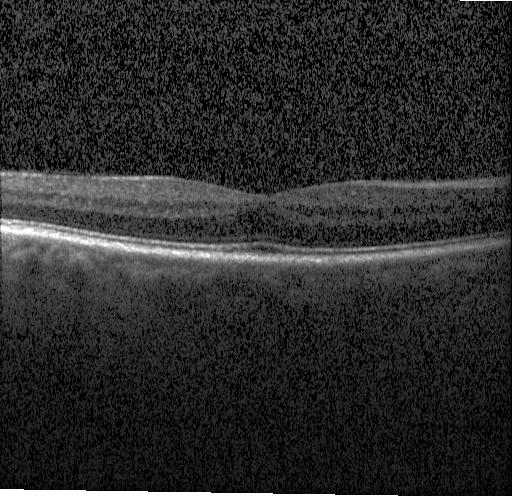 Spectral-domain optical coherence tomography; optical coherence tomography scan
Assessment: no choroidal neovascularization, diabetic macular edema, or drusen.